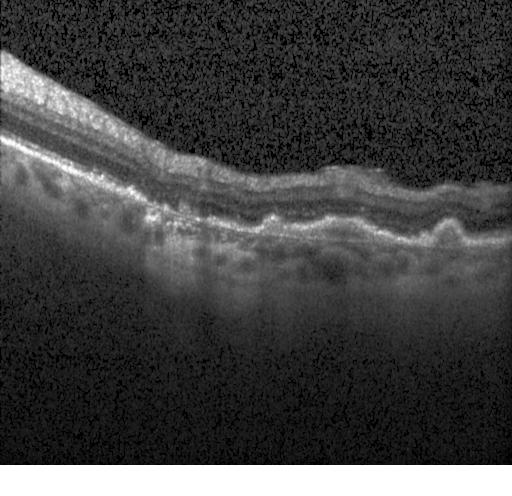
Spectral-domain optical coherence tomography, OCT line scan. Dx: a choroidal neovascular membrane.